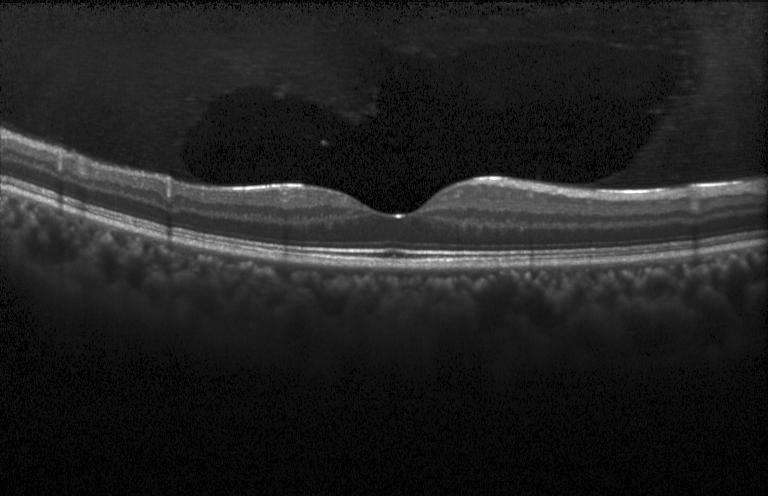

Optical coherence tomography scan — Macular OCT: no evidence of choroidal neovascularization, diabetic macular edema, or drusen.